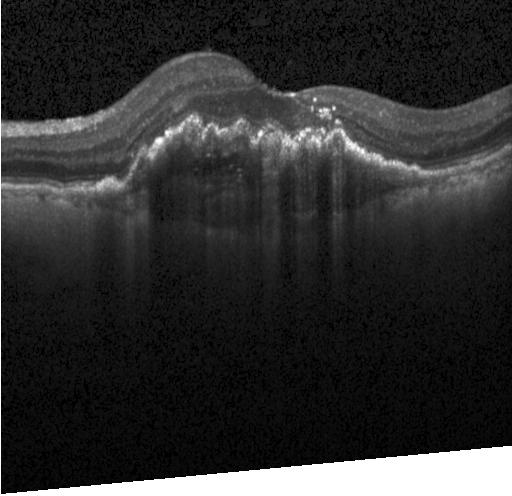

Macular OCT demonstrating choroidal neovascularization.